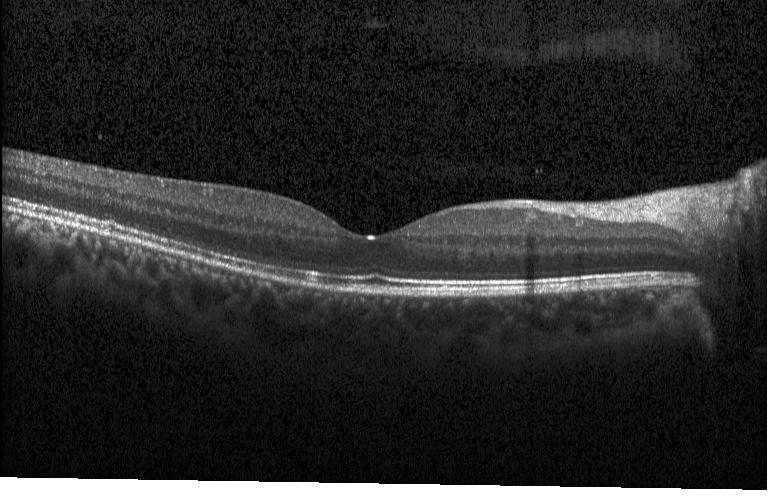
The scan shows no choroidal neovascularization, diabetic macular edema, or drusen.